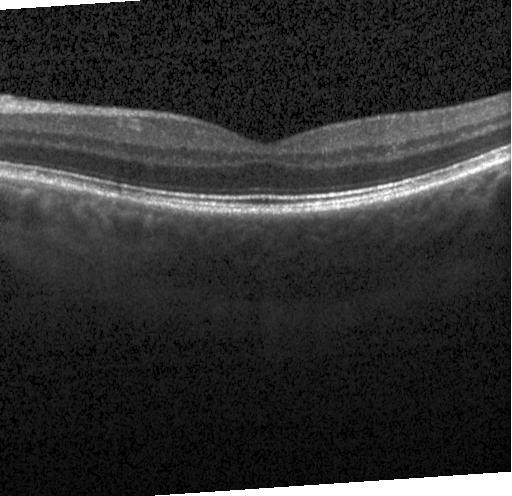
Horizontal scan through the fovea; optical coherence tomography scan; Heidelberg Spectralis OCT system; spectral-domain OCT
Diagnosis: neither CNV, DME, nor drusen.